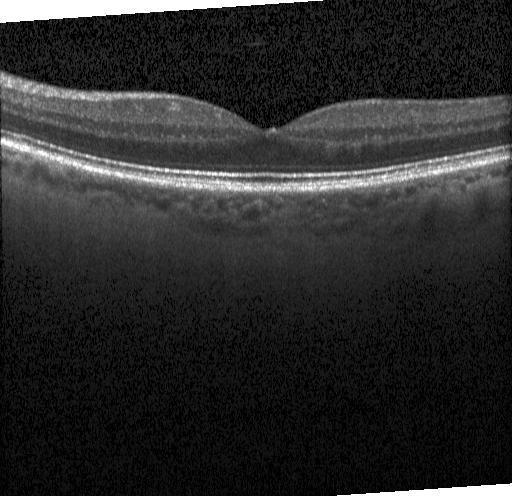 The scan shows no evidence of choroidal neovascularization, diabetic macular edema, or drusen.